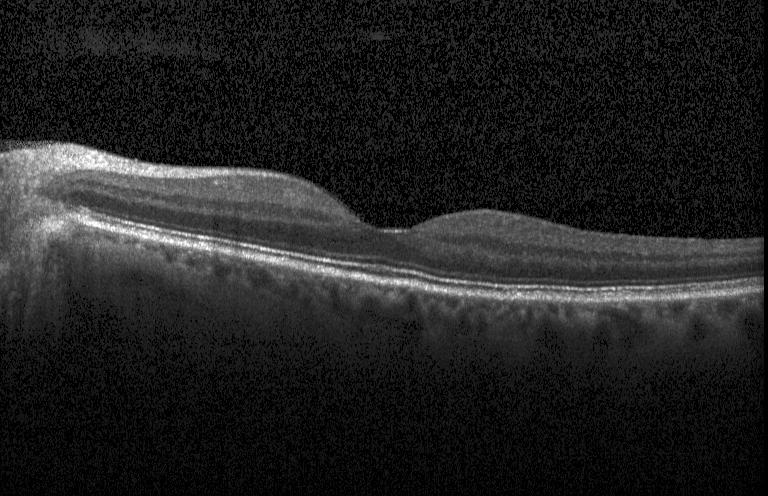

The scan shows neither choroidal neovascularization, diabetic macular edema, nor drusen.